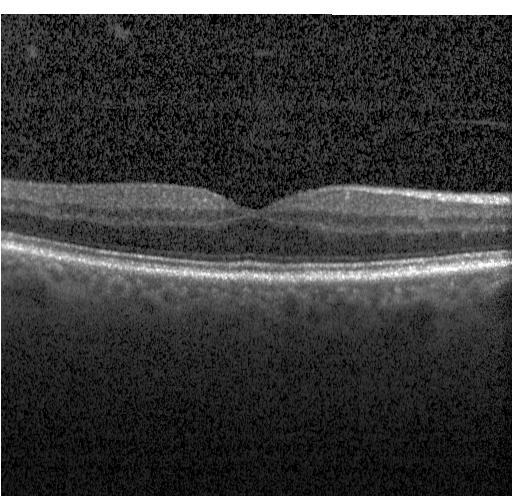
SD-OCT. Horizontal scan through the fovea. Heidelberg Spectralis OCT system. Retinal OCT B-scan
Finding: no choroidal neovascularization, no diabetic macular edema, and no drusen.